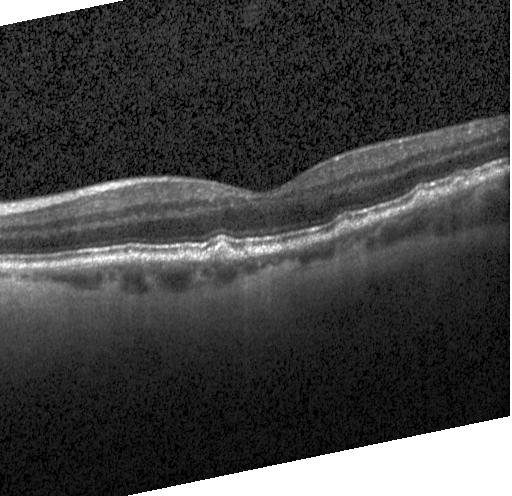

Retinal OCT cross-section · instrument: Heidelberg Spectralis · spectral-domain OCT.
The scan shows drusen.